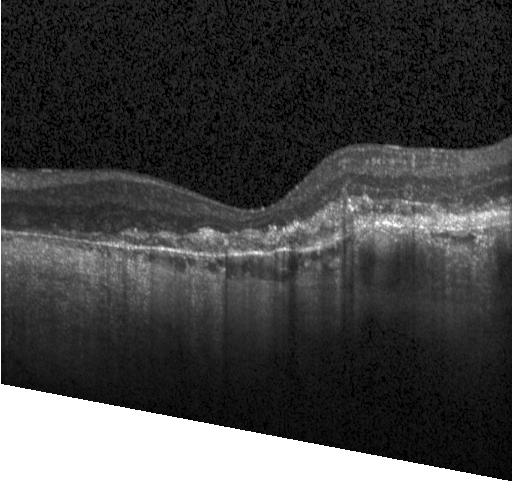 Optical coherence tomography B-scan
Impression: a choroidal neovascular membrane.